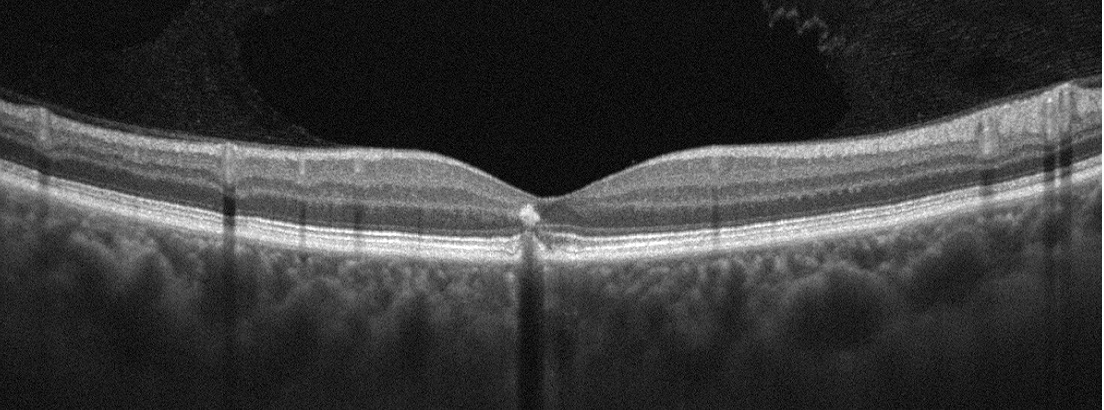
Acquired on an Optovue Avanti RTVue XR; OCT line scan; through the macula. Age-related macular degeneration (AMD).